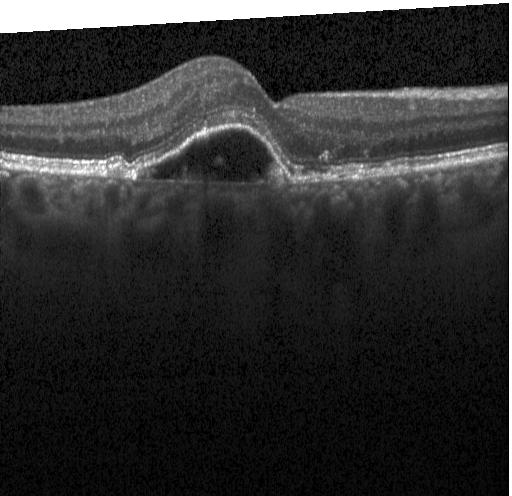

Impression: a choroidal neovascular membrane.